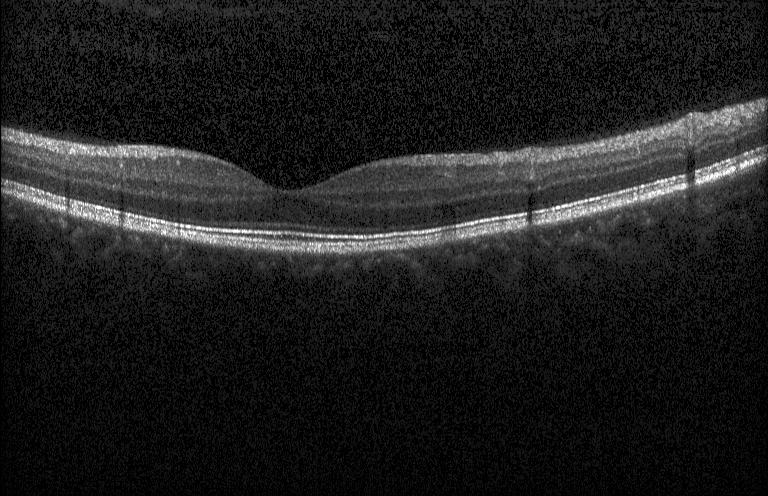
Heidelberg Spectralis OCT system. Retinal OCT cross-section
Finding: no CNV, no DME, and no drusen.